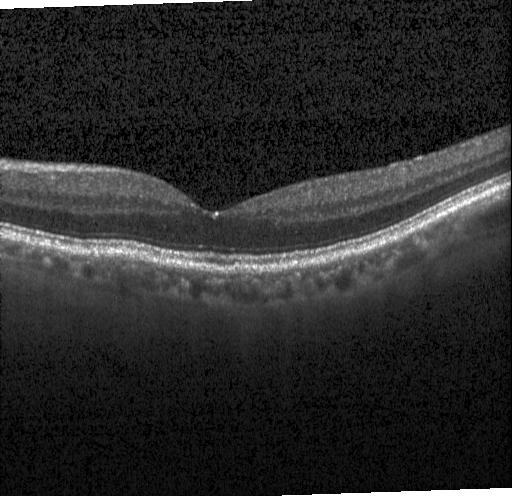

OCT line scan
OCT finding: no evidence of CNV, DME, or drusen.